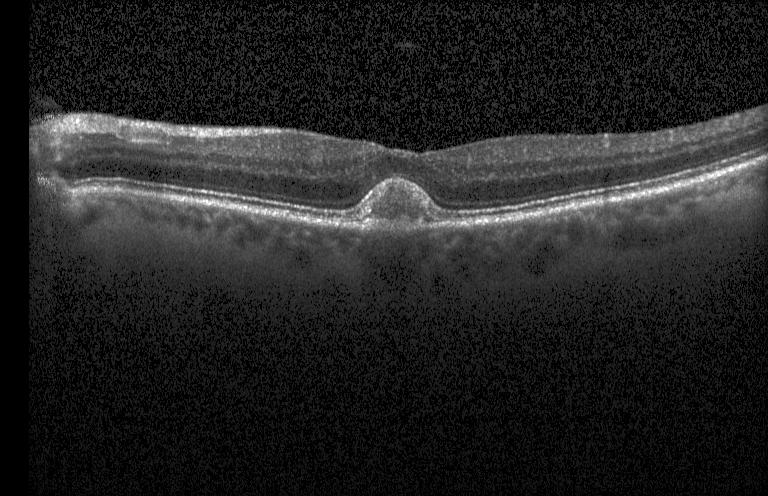

OCT B-scan showing a choroidal neovascular membrane.